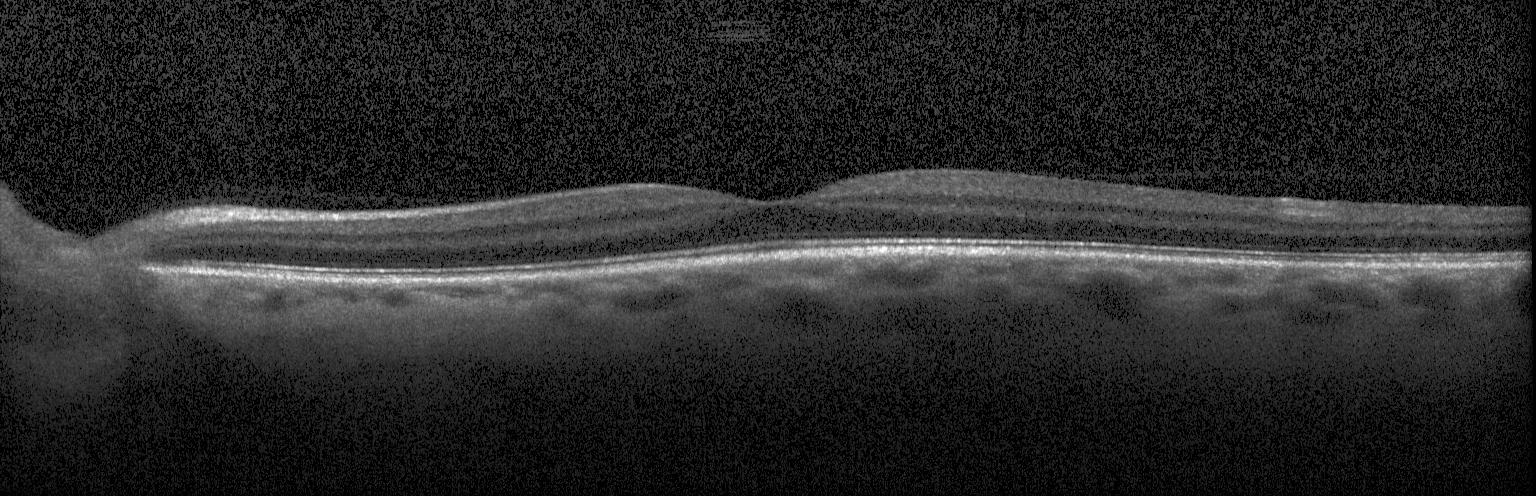

Horizontal scan through the fovea · optical coherence tomography scan · spectral-domain OCT · instrument: Heidelberg Spectralis.
OCT finding: no choroidal neovascularization, no diabetic macular edema, and no drusen.